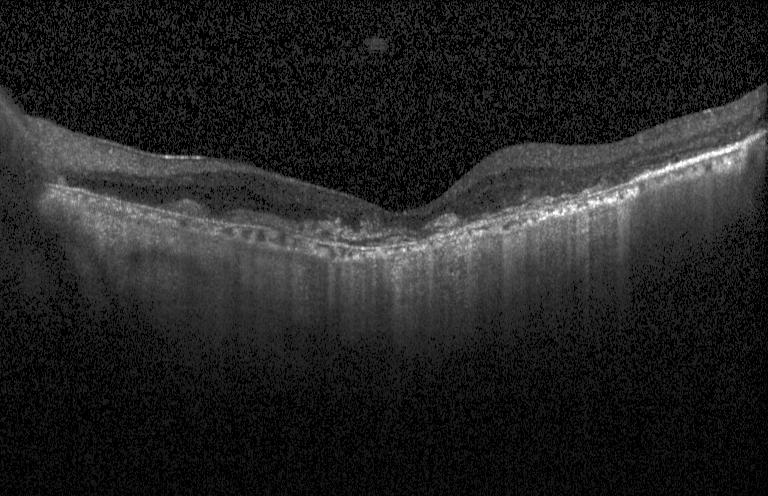
Retinal OCT cross-section — The scan shows a choroidal neovascular membrane.